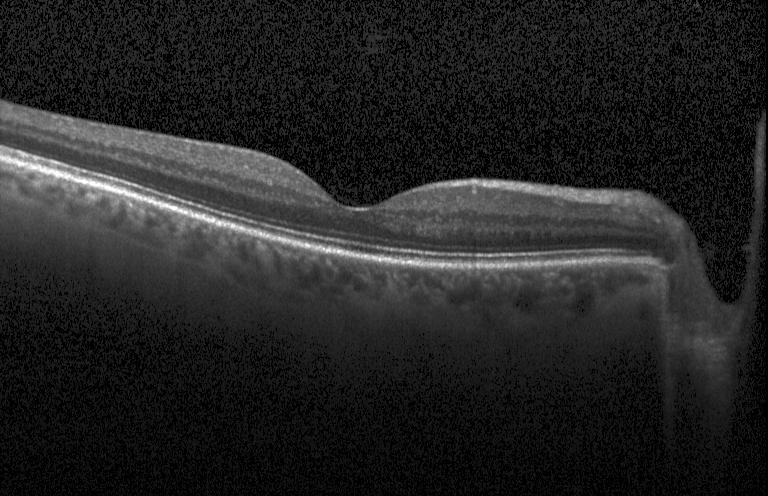 Diagnosis: no evidence of choroidal neovascularization, diabetic macular edema, or drusen.